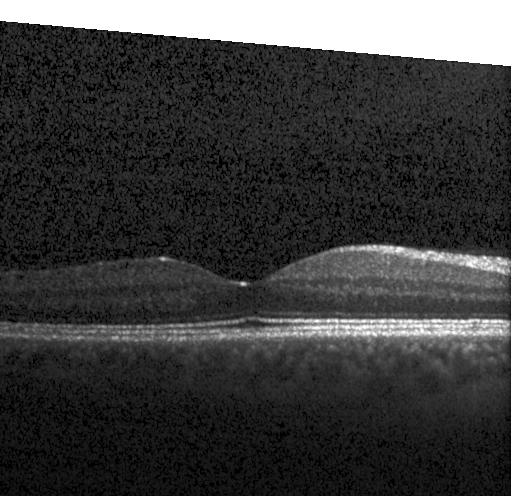 OCT line scan — Impression: neither CNV, DME, nor drusen.